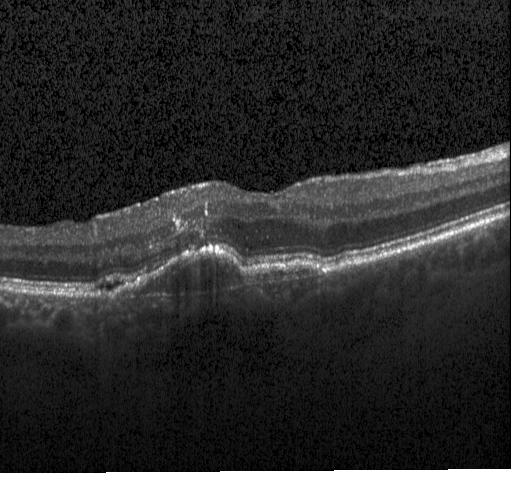 Heidelberg Spectralis OCT system · OCT B-scan · through the macula — Diagnosis: a choroidal neovascular membrane.